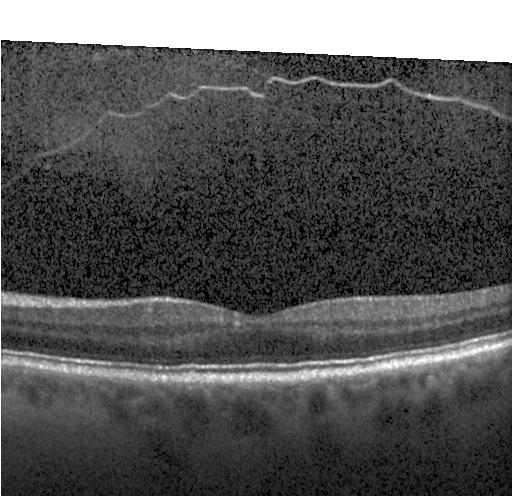

Macular OCT: no CNV, no DME, and no drusen.